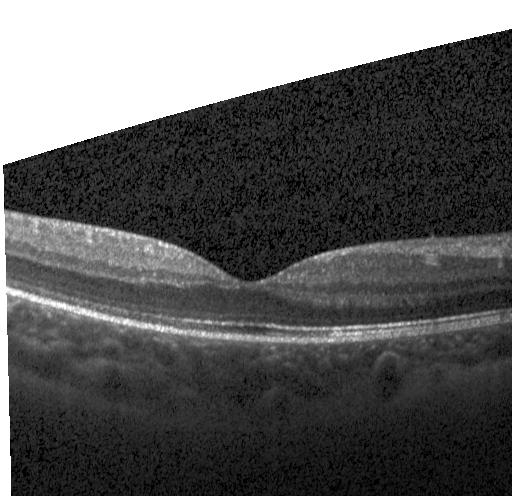

Optical coherence tomography B-scan.
Assessment: neither choroidal neovascularization, diabetic macular edema, nor drusen.